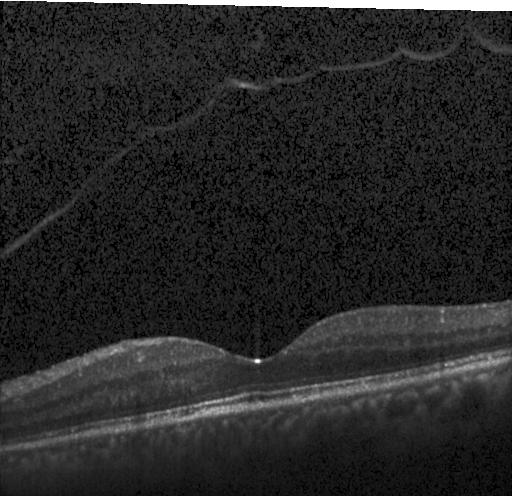
Spectral-domain OCT B-scan: neither CNV, DME, nor drusen.